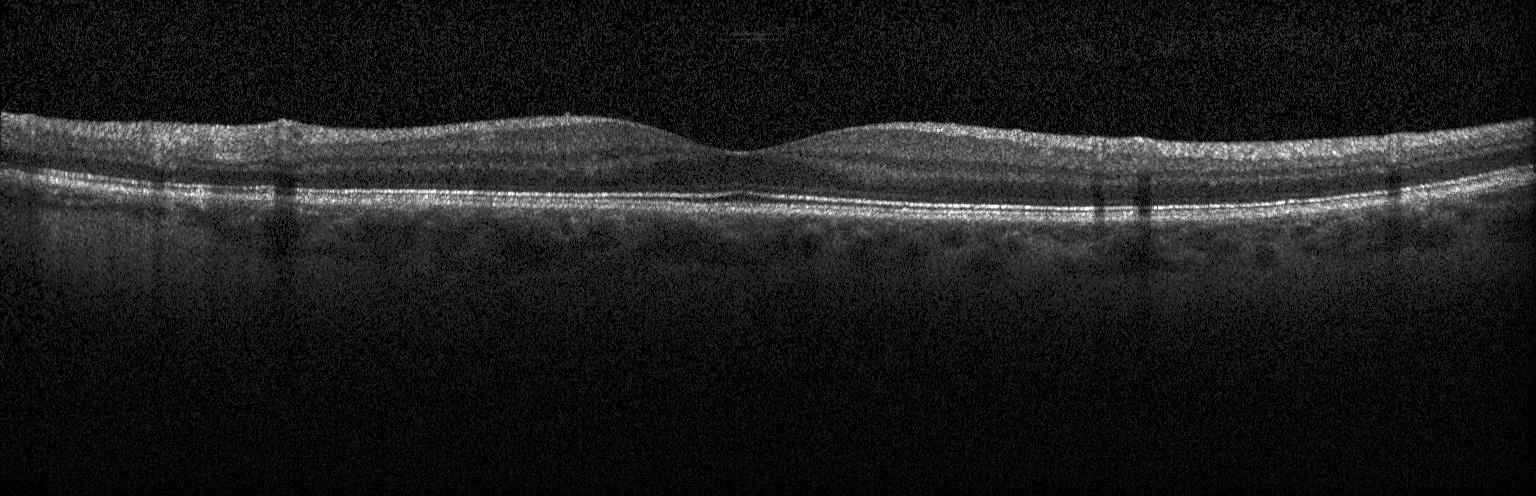
Impression: no choroidal neovascularization, diabetic macular edema, or drusen.